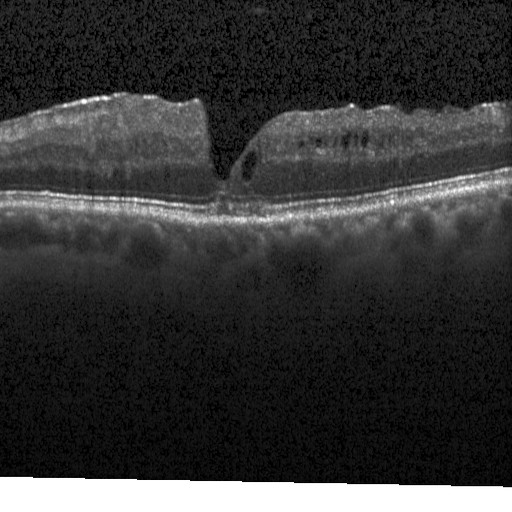 Acquired on a Heidelberg Spectralis · optical coherence tomography scan
Assessment: diabetic macular edema.